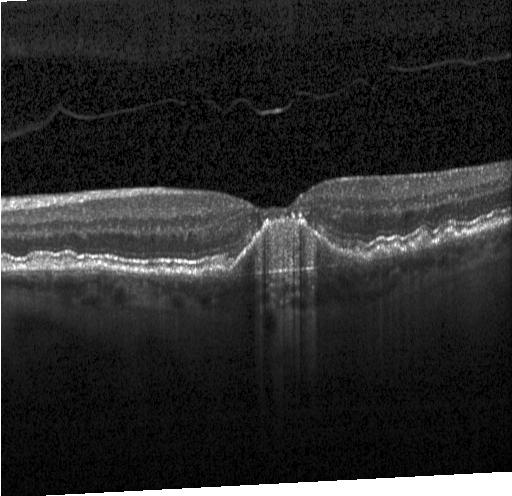

Optical coherence tomography B-scan, spectral-domain optical coherence tomography, fovea-centered. Diagnosis: a choroidal neovascular membrane.